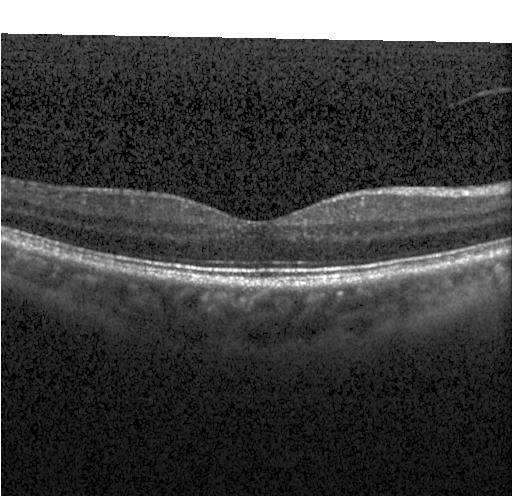
SD-OCT. Retinal OCT B-scan. Acquired on a Heidelberg Spectralis. Centered on the fovea
Finding: no CNV, no DME, and no drusen.